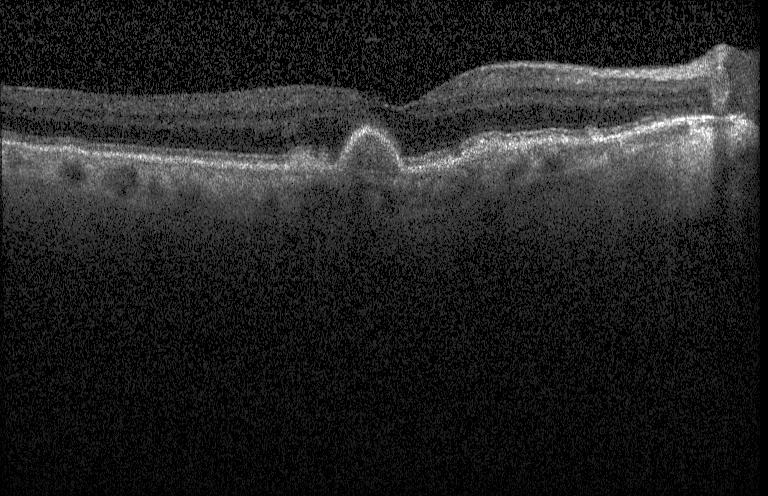 Heidelberg Spectralis, spectral-domain OCT, fovea-centered, retinal OCT B-scan — Multiple drusen.